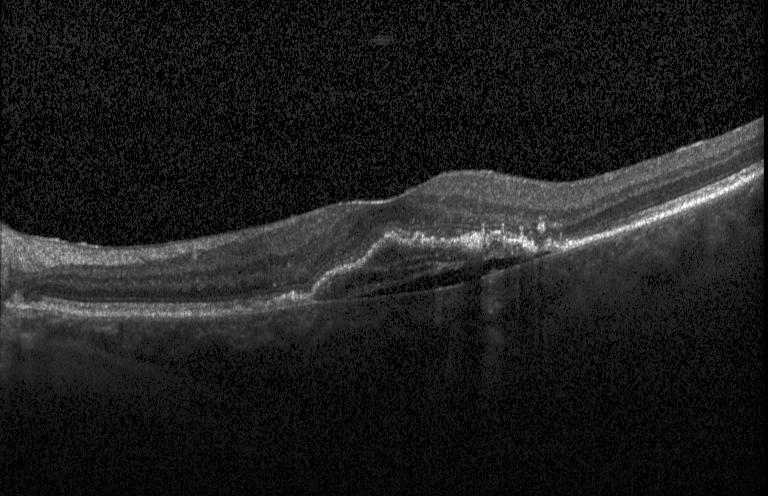

Impression: choroidal neovascularization.